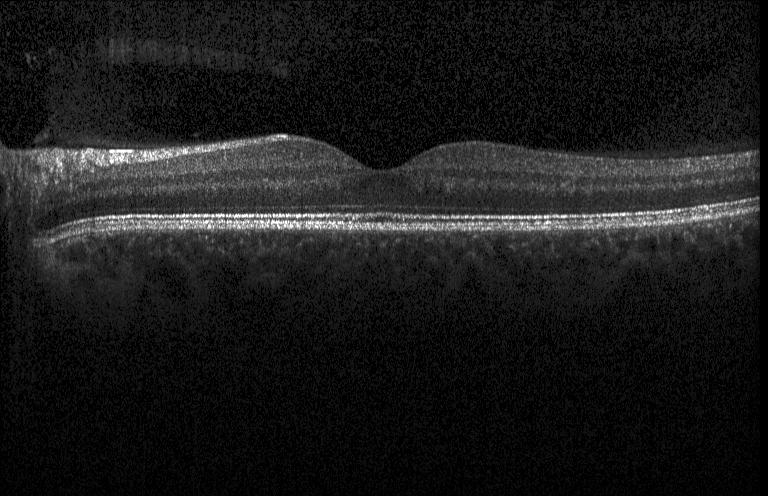 Macular scan, optical coherence tomography B-scan — Impression: no CNV, DME, or drusen.